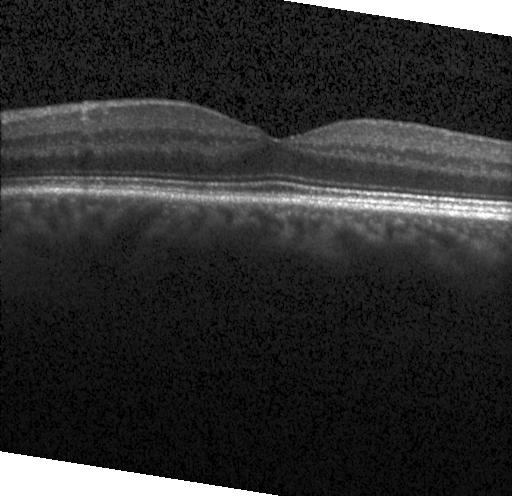

Acquired on a Heidelberg Spectralis, through the macula, SD-OCT, optical coherence tomography B-scan. The scan shows no evidence of choroidal neovascularization, diabetic macular edema, or drusen.